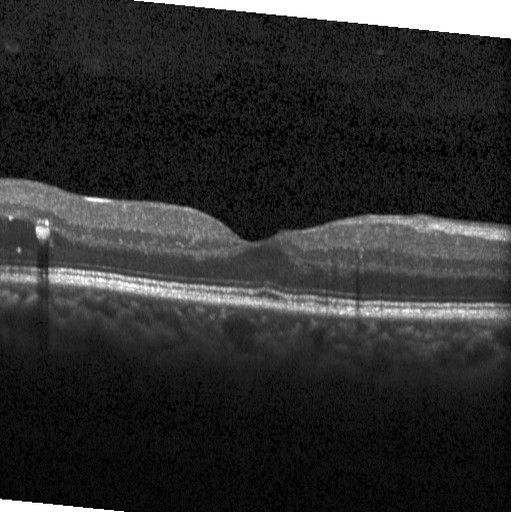

OCT B-scan. Diagnosis: DME.